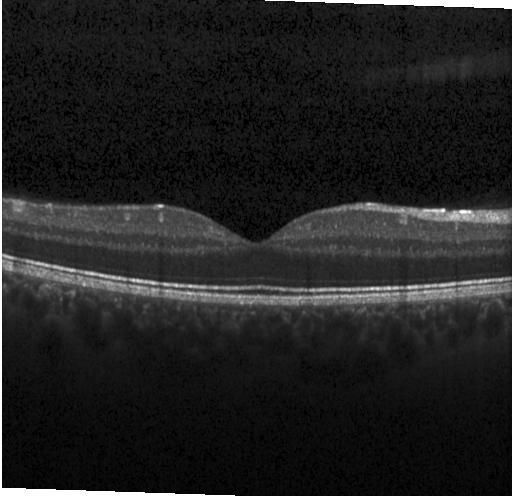

SD-OCT; OCT line scan
Impression: no choroidal neovascularization, diabetic macular edema, or drusen.